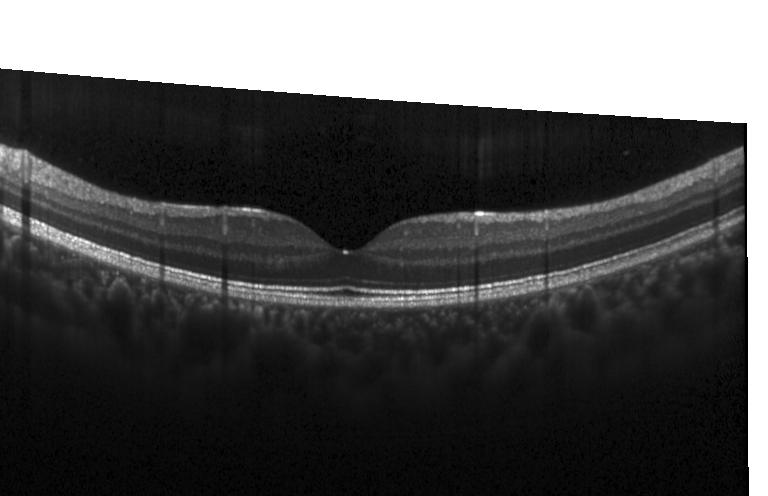 Diagnosis: neither choroidal neovascularization, diabetic macular edema, nor drusen.